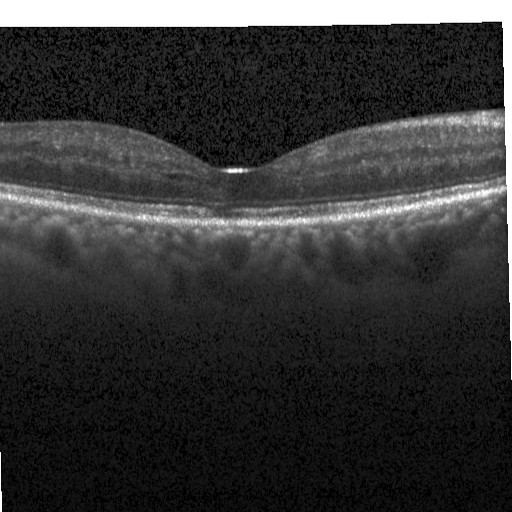 OCT line scan — Assessment: diabetic macular edema.